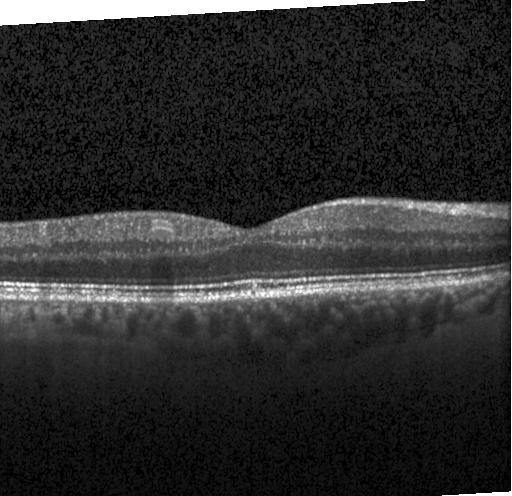

This B-scan demonstrates no choroidal neovascularization, diabetic macular edema, or drusen.